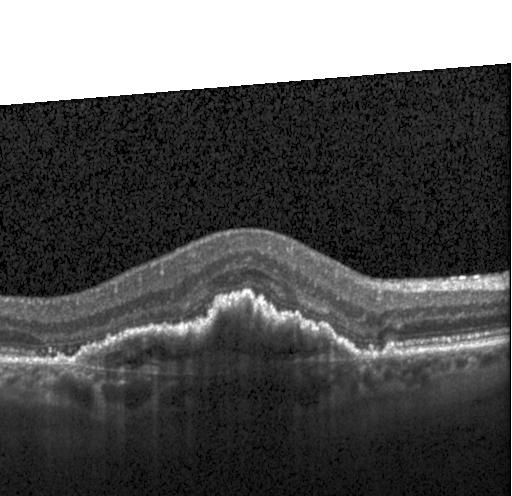 Instrument: Heidelberg Spectralis · OCT line scan · centered on the fovea · spectral-domain optical coherence tomography. This B-scan demonstrates CNV.